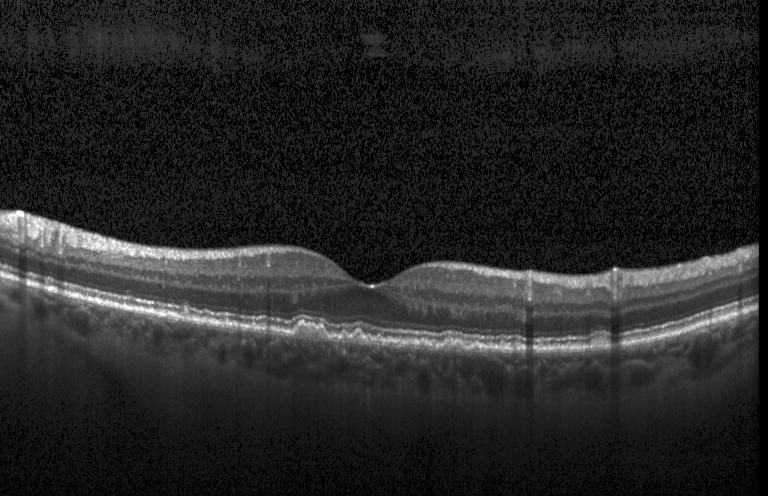

Spectral-domain optical coherence tomography. Instrument: Heidelberg Spectralis. Fovea-centered. Optical coherence tomography scan. Dx: multiple drusen.